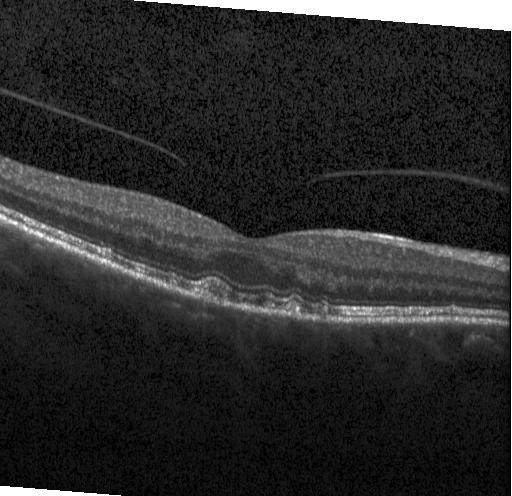

Through the macula, Heidelberg Spectralis OCT system, OCT line scan. Impression: drusen.